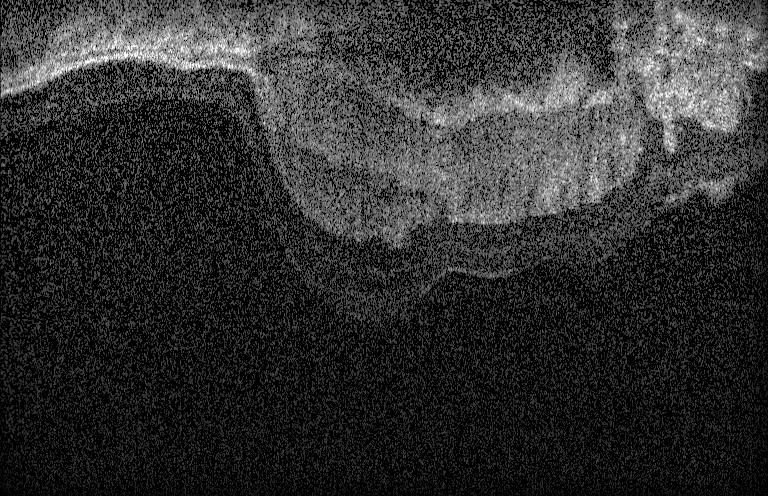
This B-scan demonstrates choroidal neovascularization (CNV).